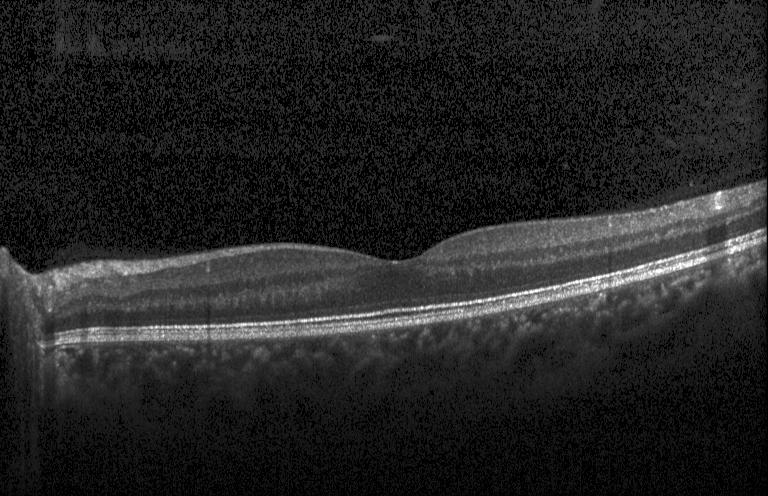 Retinal OCT cross-section showing neither CNV, DME, nor drusen.